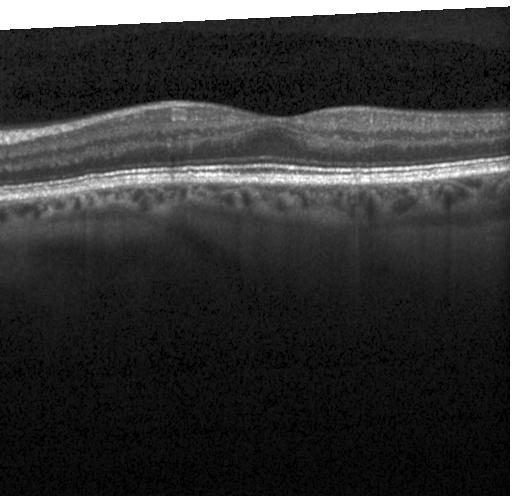

Optical coherence tomography B-scan. Spectral-domain optical coherence tomography
The scan shows no choroidal neovascularization, diabetic macular edema, or drusen.